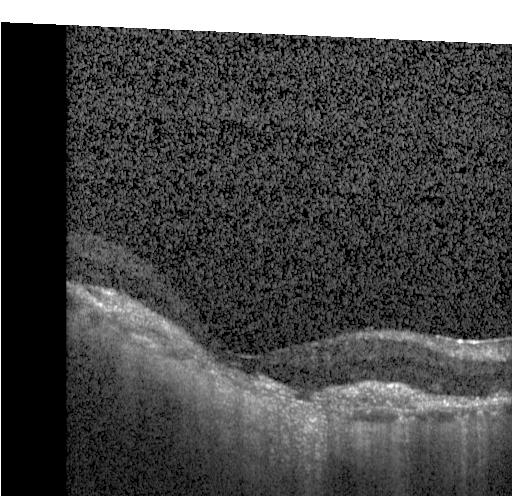 OCT scan showing a choroidal neovascular membrane.